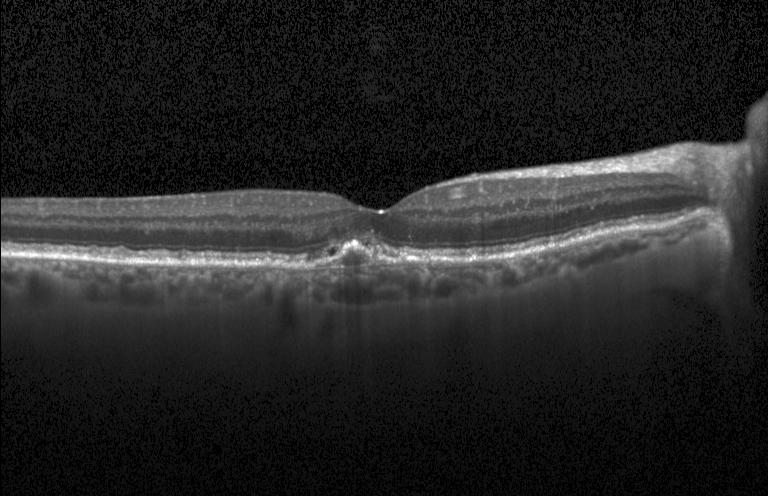 OCT finding: choroidal neovascularization.